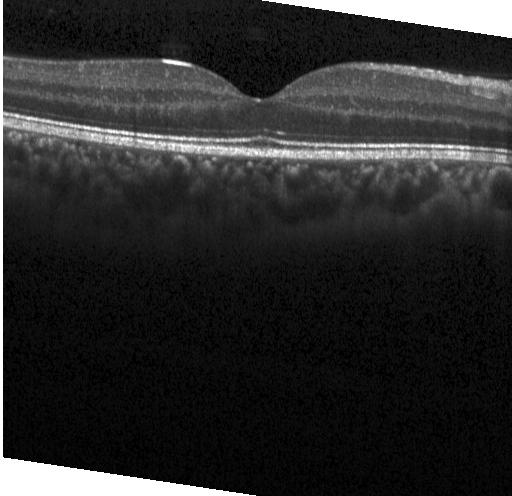 This B-scan demonstrates no choroidal neovascularization, diabetic macular edema, or drusen.